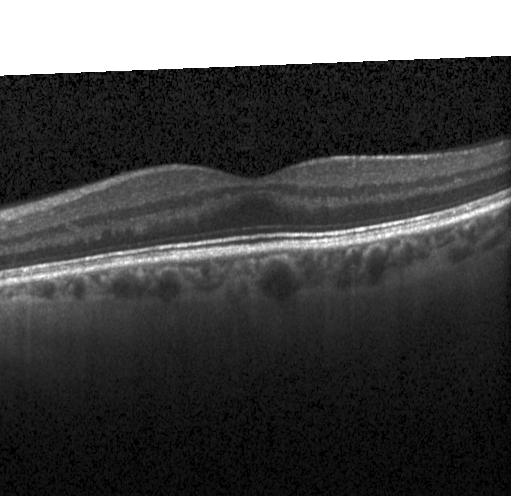

OCT line scan
Diagnosis: neither CNV, DME, nor drusen.